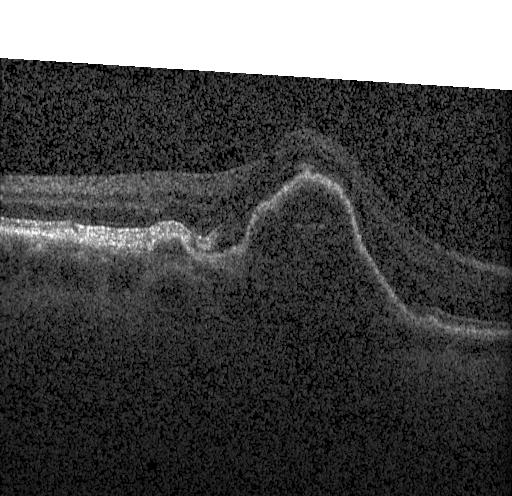

Diagnosis: choroidal neovascularization (CNV).